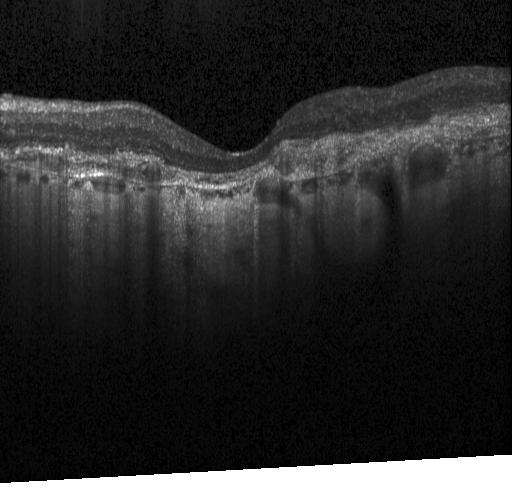

Diagnosis: a choroidal neovascular membrane.